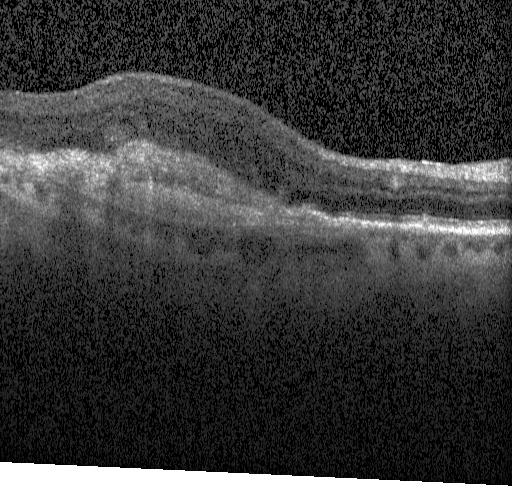 Spectral-domain optical coherence tomography. Retinal OCT B-scan. A choroidal neovascular membrane.